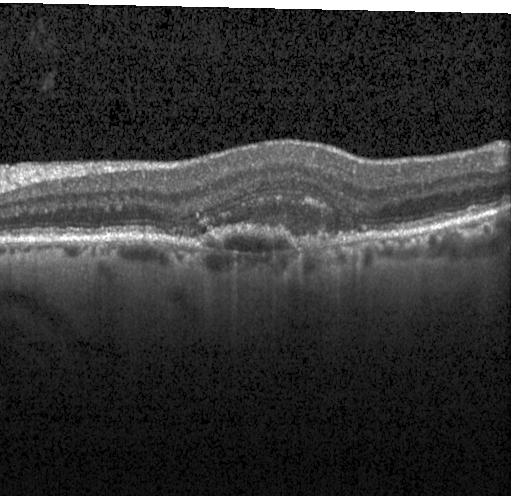

Optical coherence tomography scan. Finding: choroidal neovascularization.